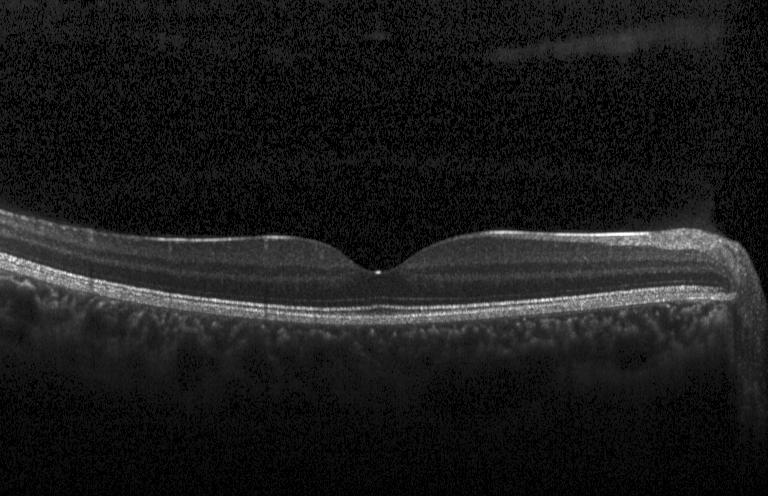

Impression: neither choroidal neovascularization, diabetic macular edema, nor drusen.